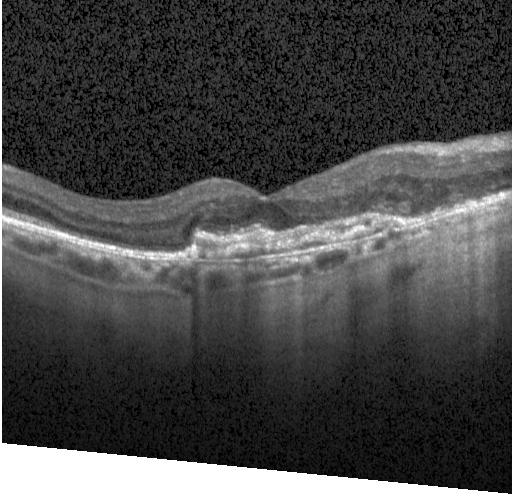 Spectral-domain optical coherence tomography. Fovea-centered. Heidelberg Spectralis. Optical coherence tomography scan.
Choroidal neovascularization (CNV).